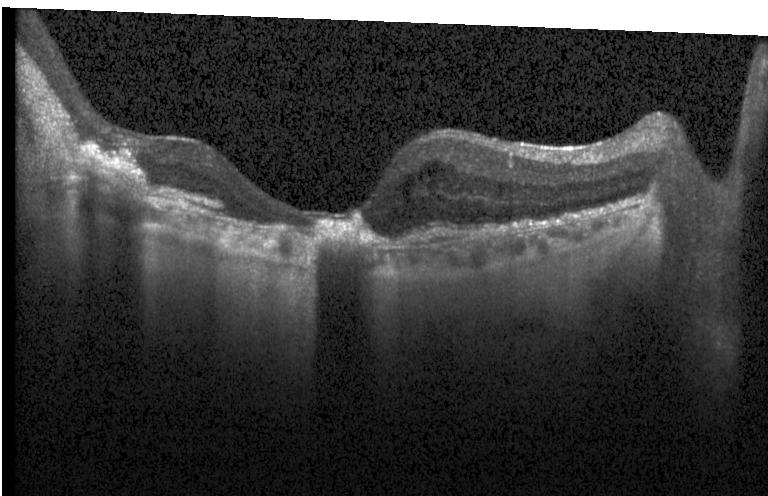
SD-OCT · fovea-centered · optical coherence tomography B-scan · Heidelberg Spectralis OCT system
Finding: a choroidal neovascular membrane.